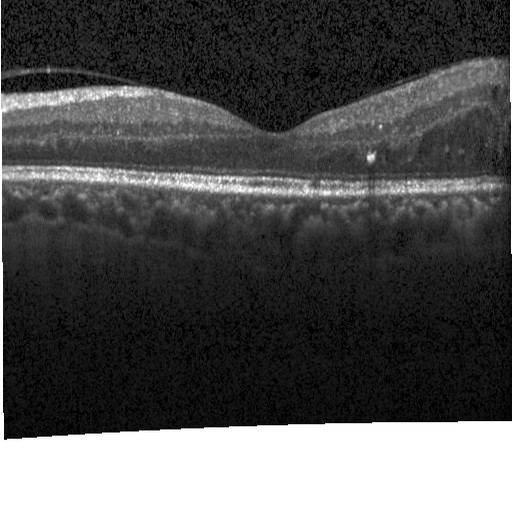 Fovea-centered, Heidelberg Spectralis, optical coherence tomography scan, spectral-domain OCT.
Assessment: diabetic macular edema (DME).